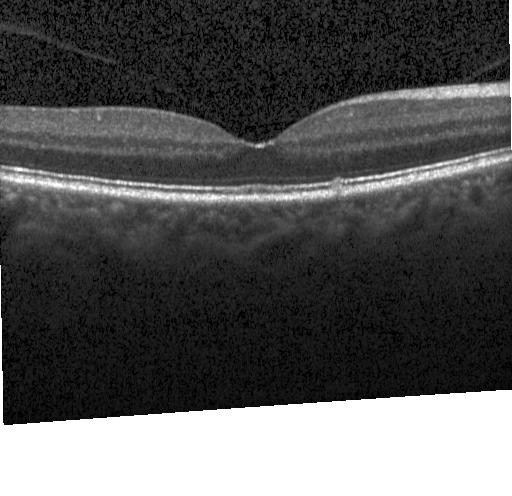 Heidelberg Spectralis OCT system, retinal OCT B-scan, spectral-domain optical coherence tomography, centered on the fovea. Macular OCT: drusen.